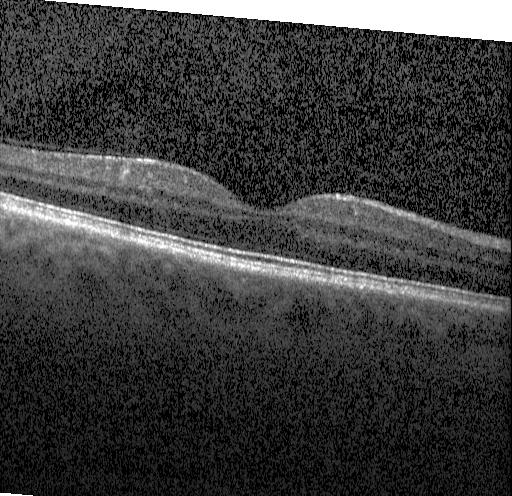

Through the macula · optical coherence tomography B-scan. Macular OCT: no evidence of CNV, DME, or drusen.